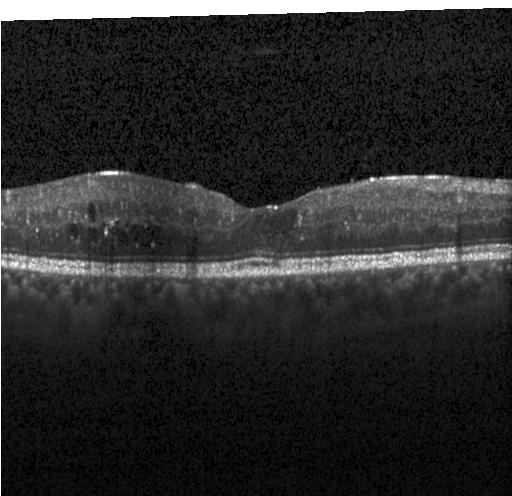 Impression: DME.